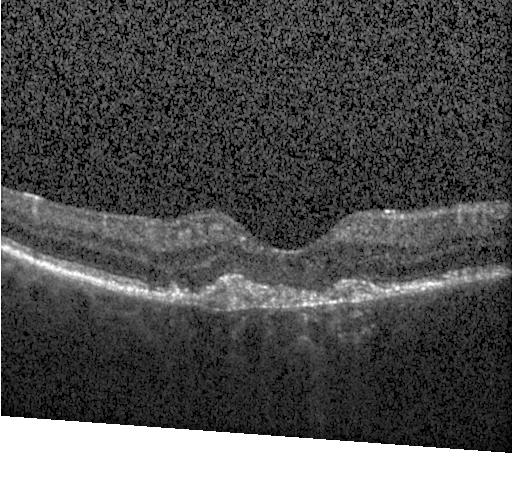
Diagnosis: choroidal neovascularization.